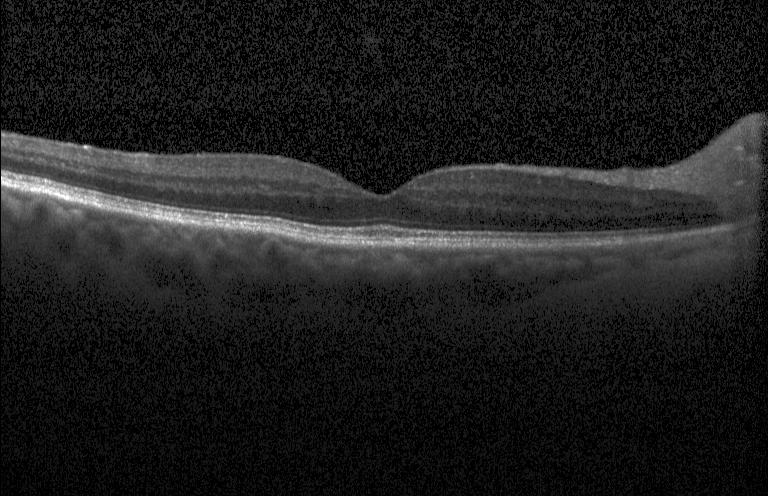 Optical coherence tomography B-scan, SD-OCT — OCT finding: no evidence of CNV, DME, or drusen.